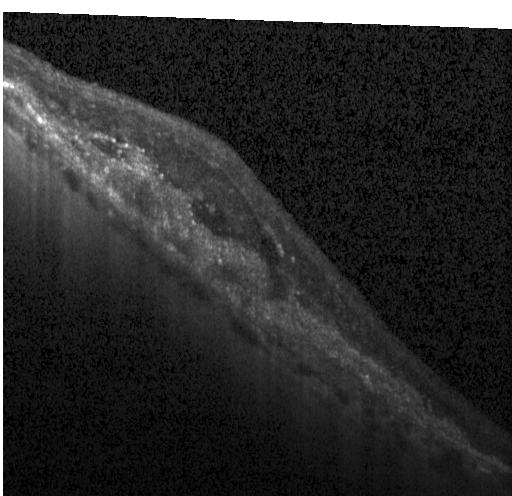
Spectral-domain optical coherence tomography. Optical coherence tomography scan. Fovea-centered. Heidelberg Spectralis OCT system.
This B-scan demonstrates a choroidal neovascular membrane.